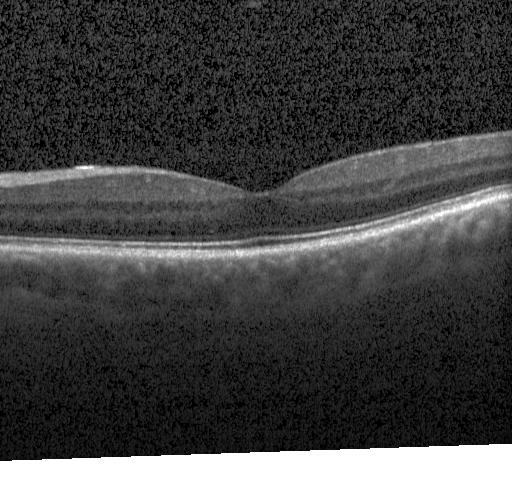
Spectral-domain OCT. OCT B-scan
Finding: no evidence of choroidal neovascularization, diabetic macular edema, or drusen.